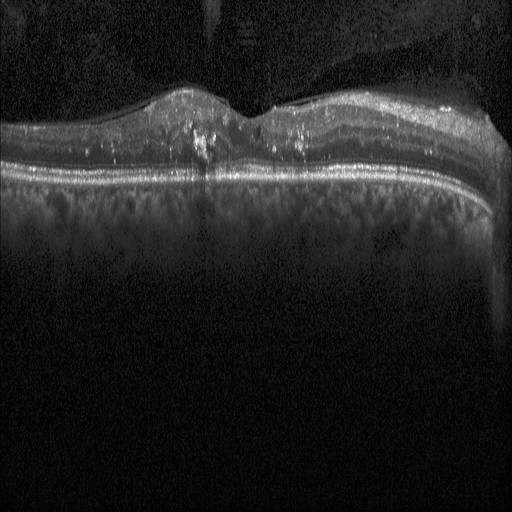

Retinal OCT B-scan — Finding: diabetic macular edema (DME).